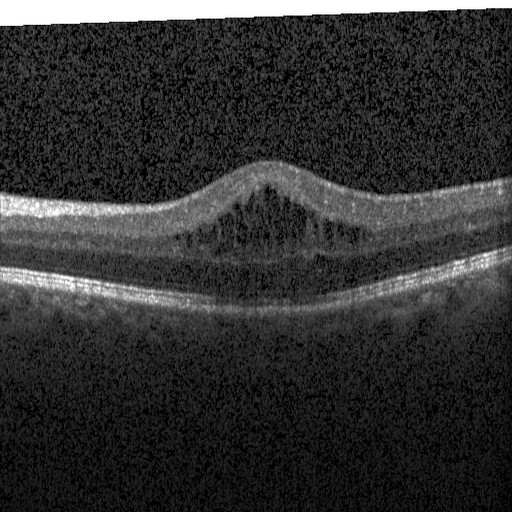 Diagnosis: diabetic macular edema (DME).